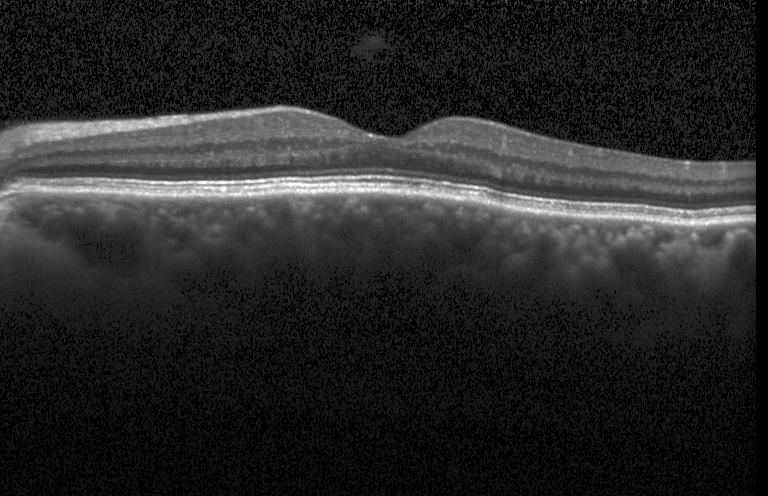
Impression: no CNV, no DME, and no drusen.